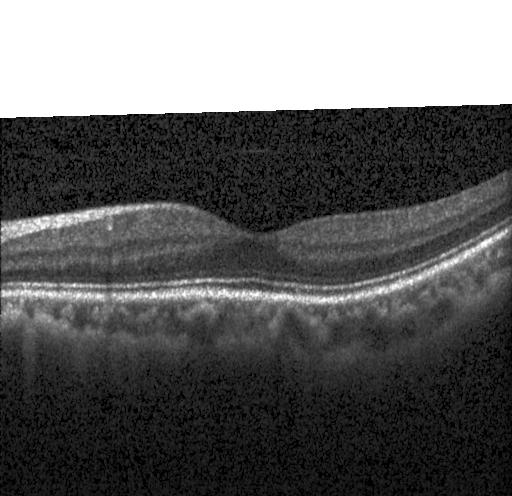 OCT B-scan
Assessment: neither choroidal neovascularization, diabetic macular edema, nor drusen.